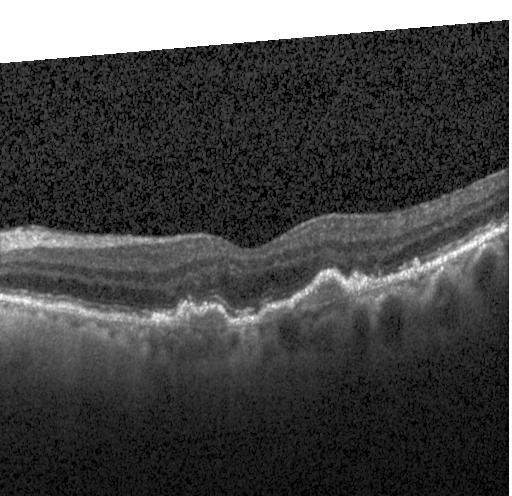

OCT line scan. This B-scan demonstrates choroidal neovascularization (CNV).